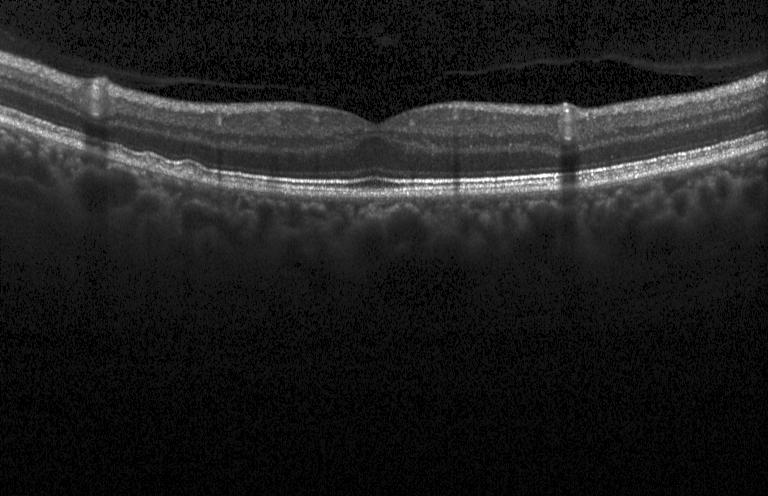
Optical coherence tomography scan; SD-OCT; horizontal scan through the fovea; Heidelberg Spectralis OCT system. OCT finding: sub-RPE drusenoid deposits.